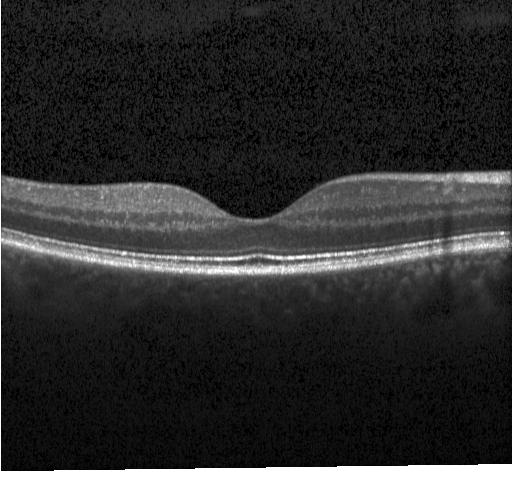 This B-scan demonstrates no evidence of CNV, DME, or drusen.